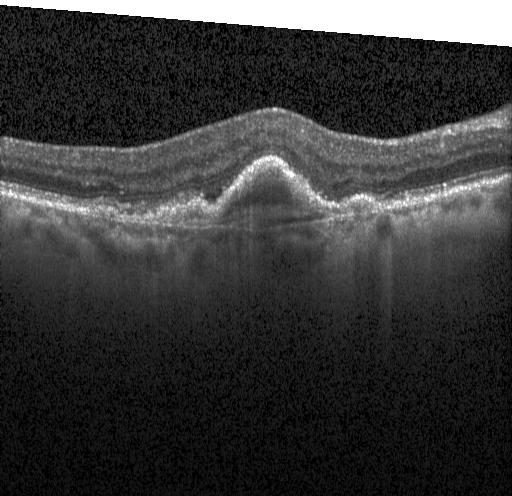

Retinal OCT cross-section. Heidelberg Spectralis. Spectral-domain optical coherence tomography. Centered on the fovea — This B-scan demonstrates CNV.